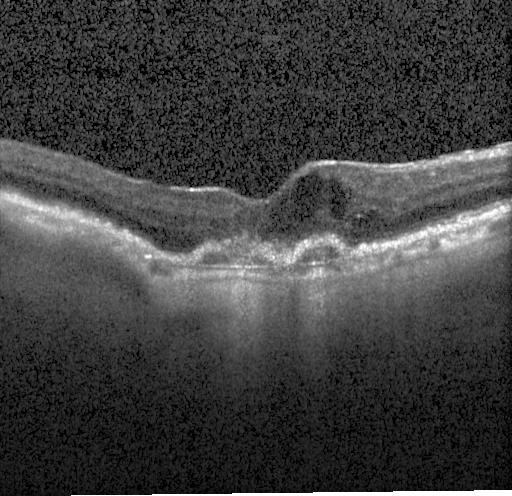

SD-OCT; optical coherence tomography B-scan; fovea-centered; Heidelberg Spectralis OCT system
Finding: choroidal neovascularization (CNV).